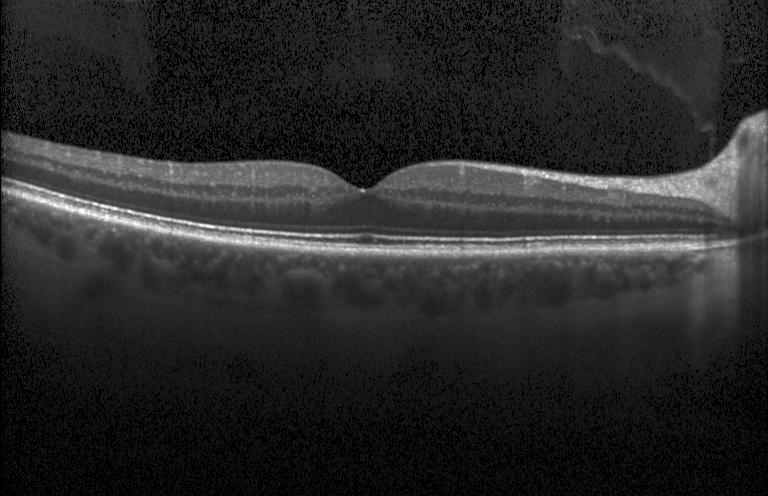

Horizontal scan through the fovea · OCT B-scan
Diagnosis: no CNV, DME, or drusen.